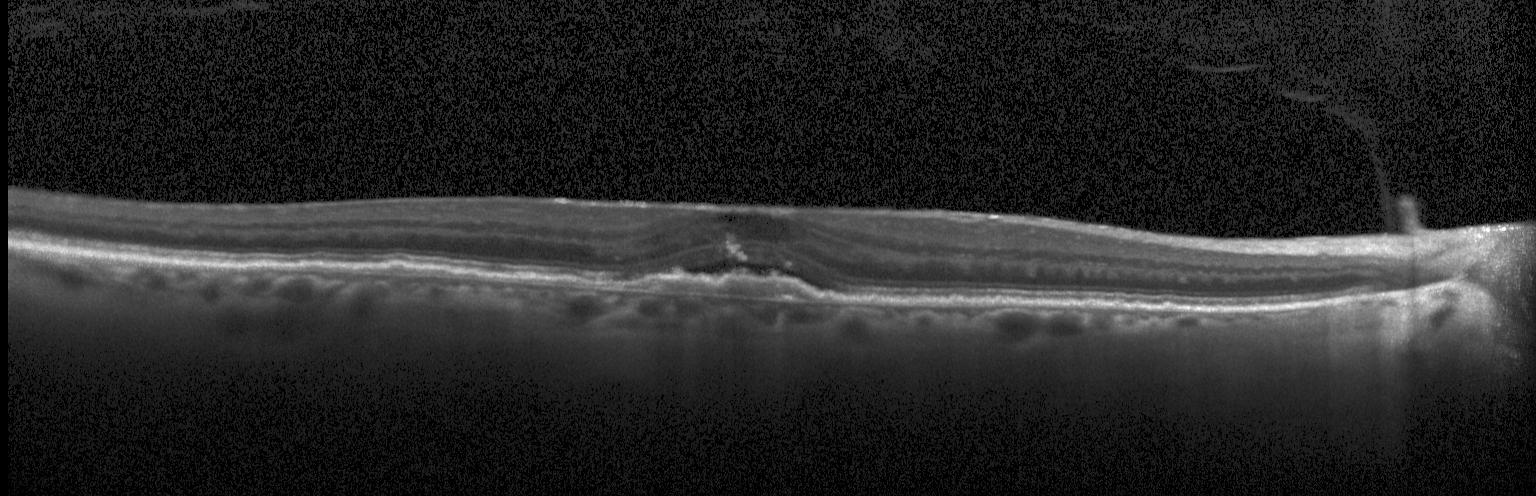
This B-scan demonstrates a choroidal neovascular membrane.